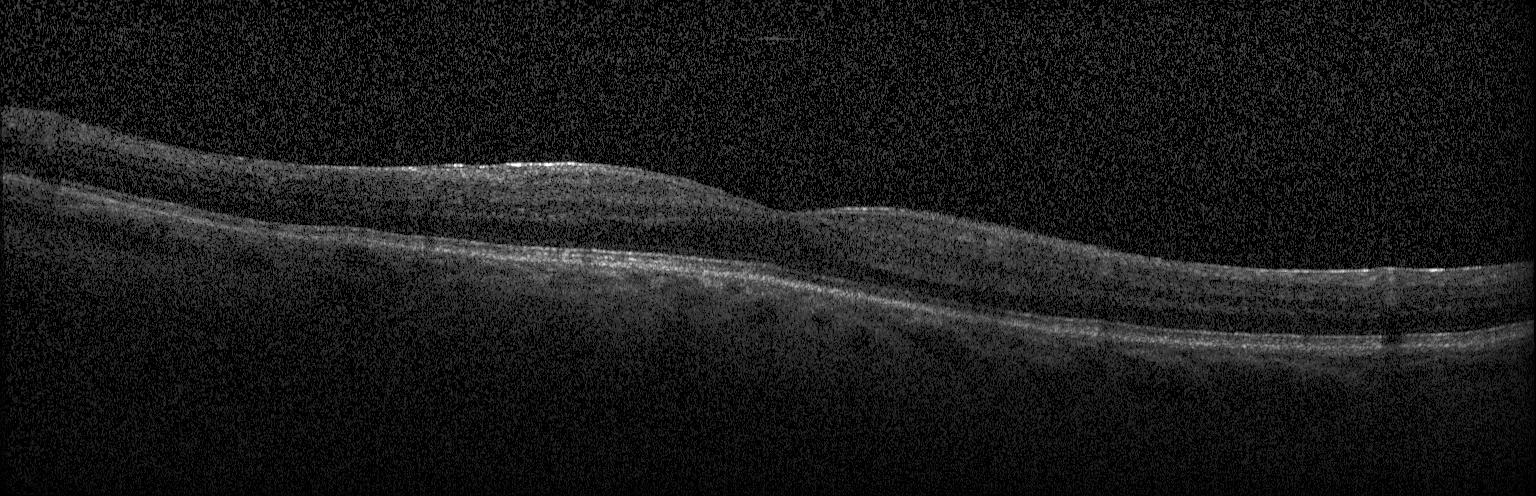 Optical coherence tomography scan — Impression: no CNV, DME, or drusen.